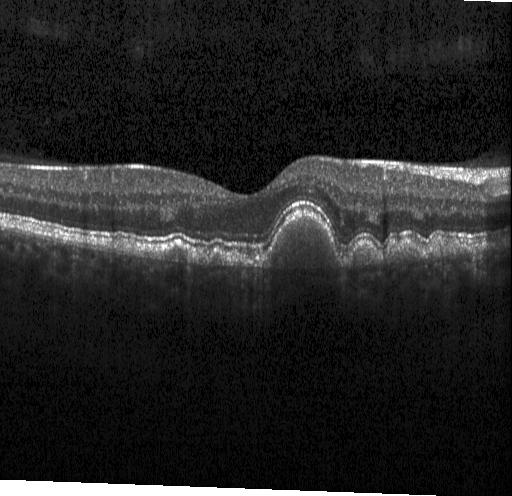
Spectral-domain OCT B-scan: multiple drusen.